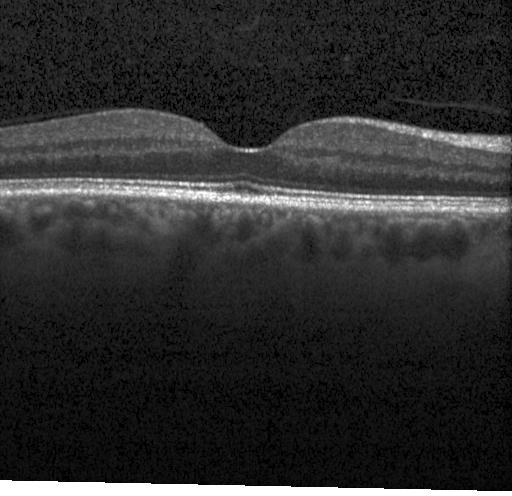

Horizontal scan through the fovea · OCT line scan. Finding: no choroidal neovascularization, diabetic macular edema, or drusen.